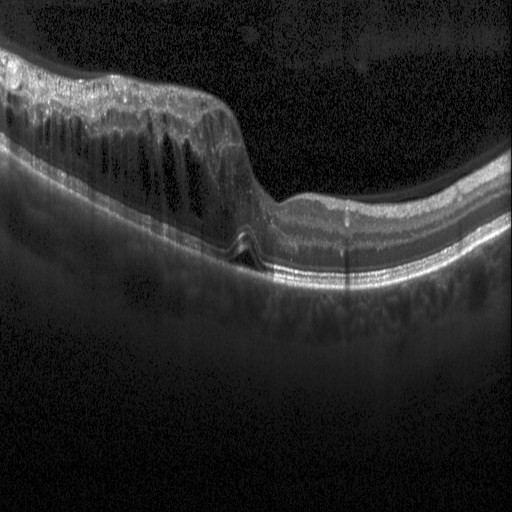

Heidelberg Spectralis; retinal OCT cross-section.
This B-scan demonstrates diabetic macular edema.